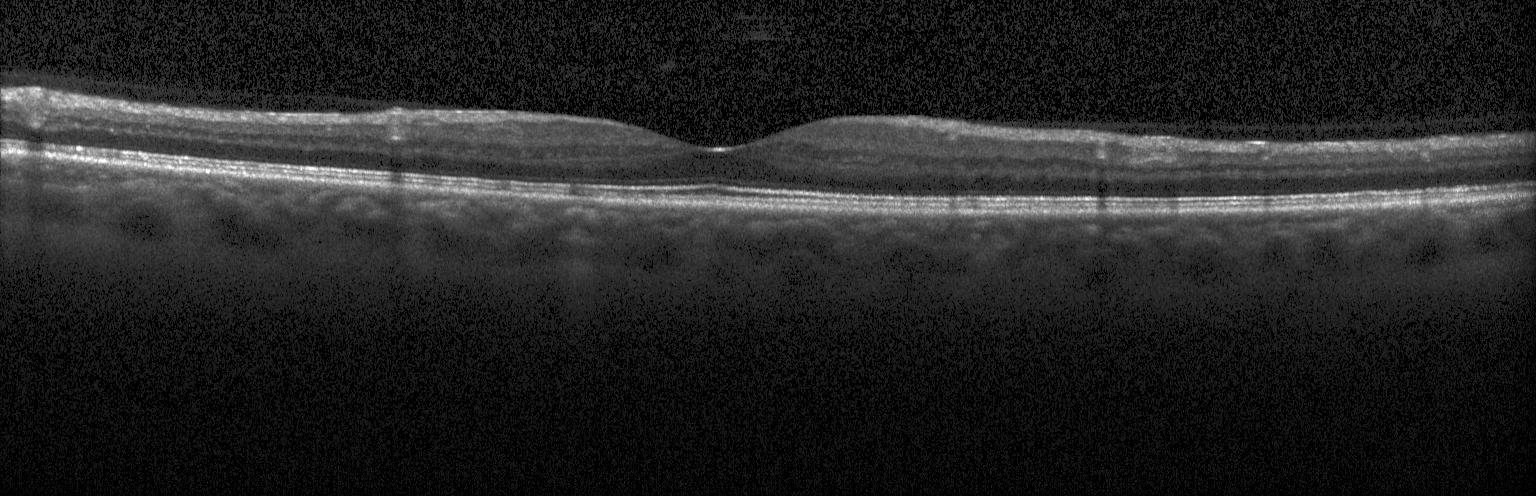

Optical coherence tomography B-scan, acquired on a Heidelberg Spectralis
Finding: no CNV, DME, or drusen.